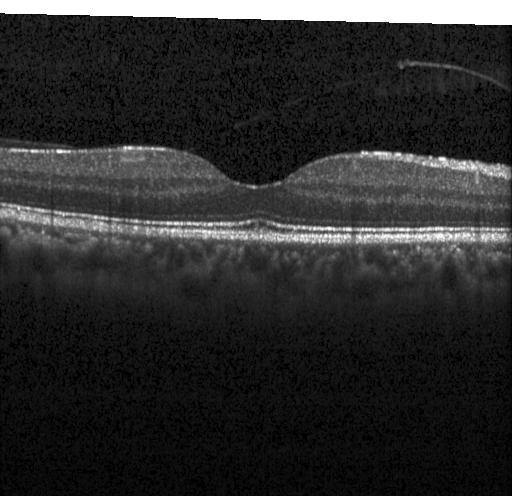

Dx: no evidence of choroidal neovascularization, diabetic macular edema, or drusen.